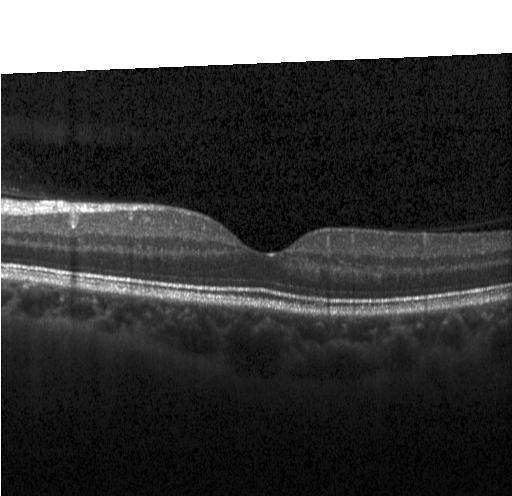

Spectral-domain OCT, Heidelberg Spectralis, OCT B-scan, through the macula.
Finding: no choroidal neovascularization, diabetic macular edema, or drusen.